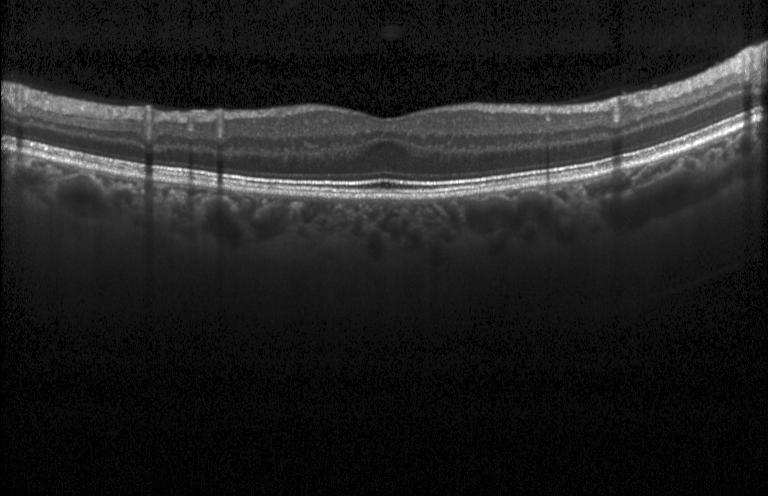
Finding: no choroidal neovascularization, no diabetic macular edema, and no drusen.